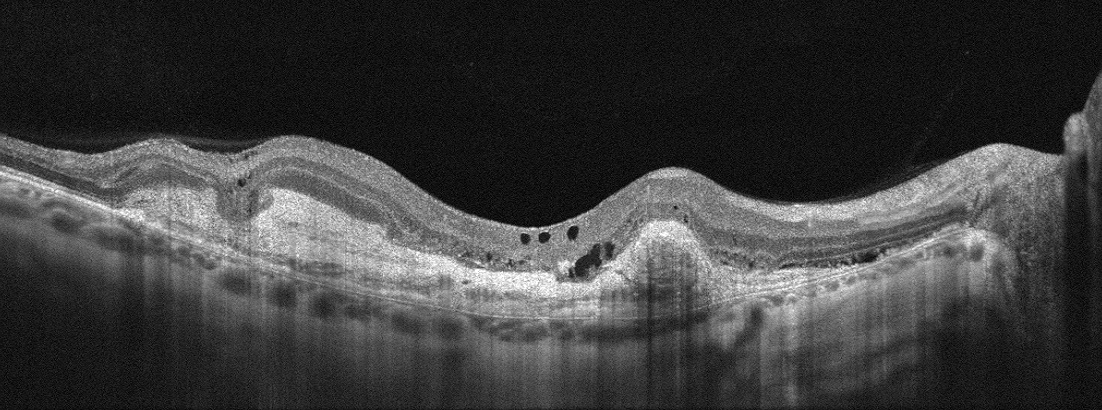
Retinal OCT cross-section. The scan shows age-related macular degeneration (AMD).